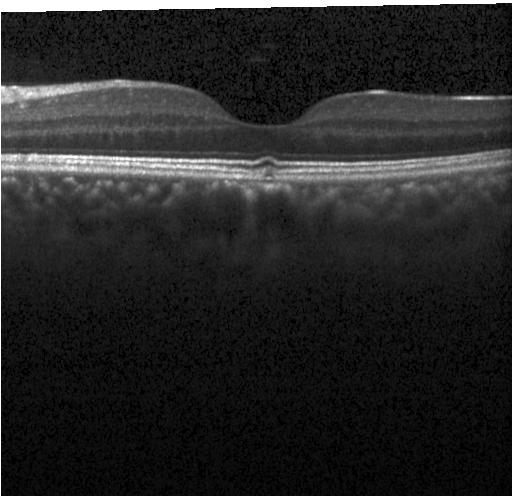

Dx: no choroidal neovascularization, diabetic macular edema, or drusen.